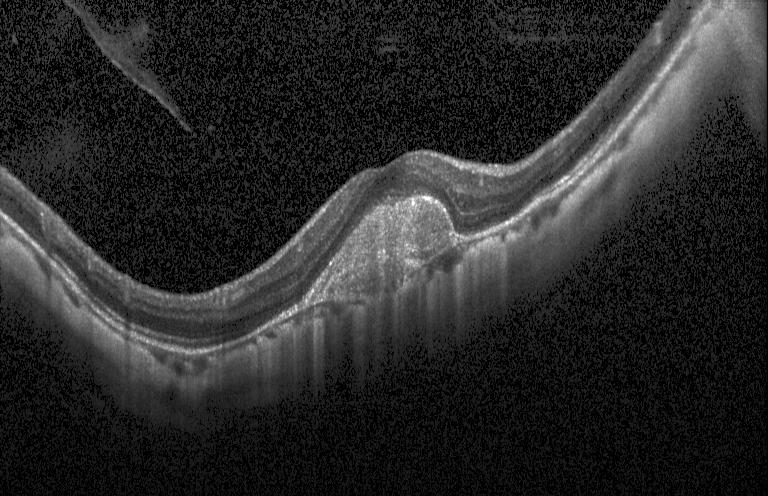

Through the macula · OCT line scan — Dx: CNV.